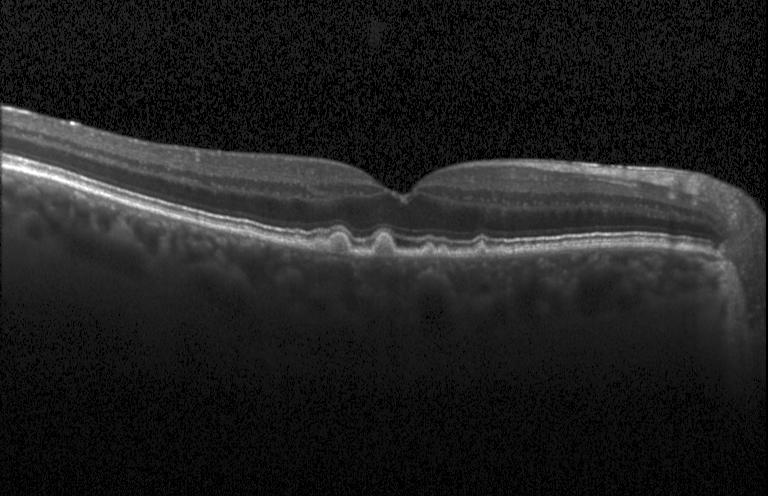 Optical coherence tomography scan; macular scan; SD-OCT. This B-scan demonstrates sub-RPE drusenoid deposits.